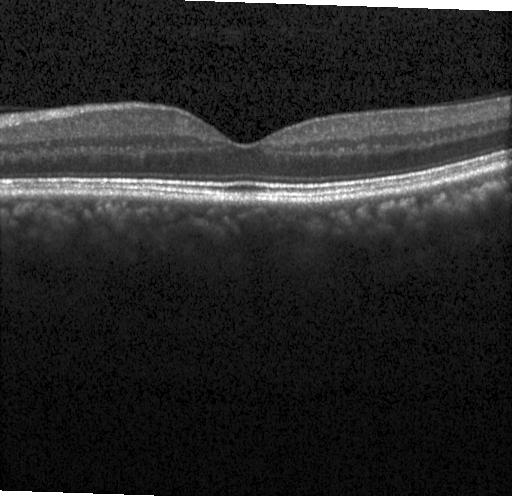
Through the macula, OCT B-scan, spectral-domain optical coherence tomography, instrument: Heidelberg Spectralis
Neither CNV, DME, nor drusen.